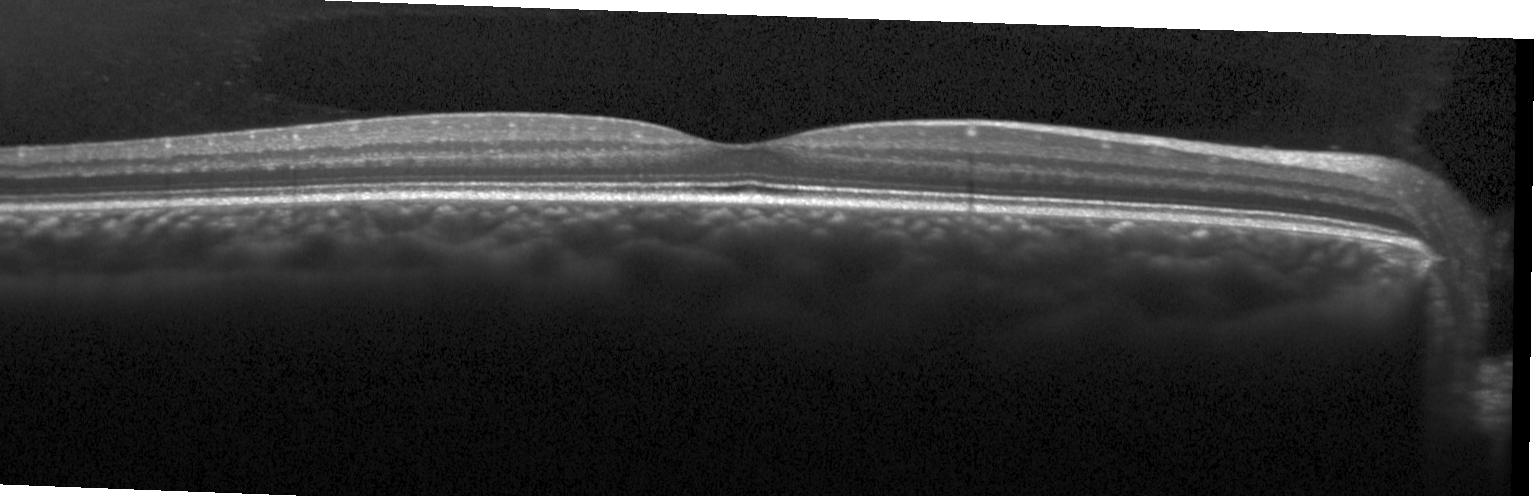

Spectral-domain OCT, optical coherence tomography B-scan. The scan shows no CNV, DME, or drusen.